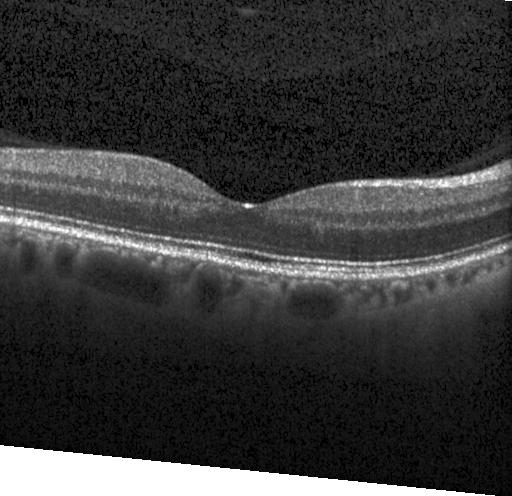
Finding: neither choroidal neovascularization, diabetic macular edema, nor drusen.